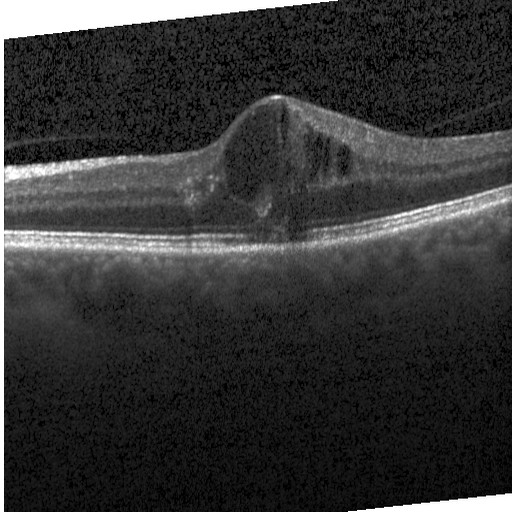

Optical coherence tomography B-scan.
Finding: diabetic macular edema (DME).